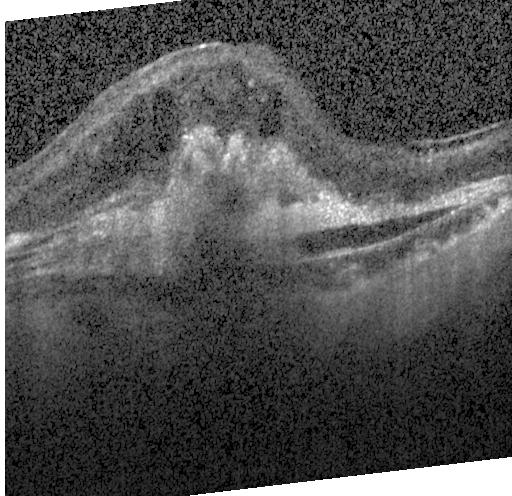 Spectral-domain OCT, instrument: Heidelberg Spectralis, macular scan, retinal OCT B-scan — This B-scan demonstrates choroidal neovascularization (CNV).